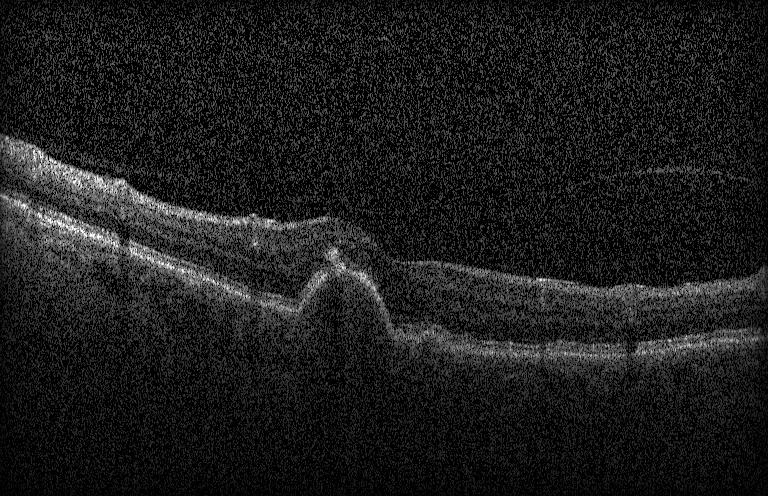 Fovea-centered · optical coherence tomography B-scan — Impression: choroidal neovascularization.